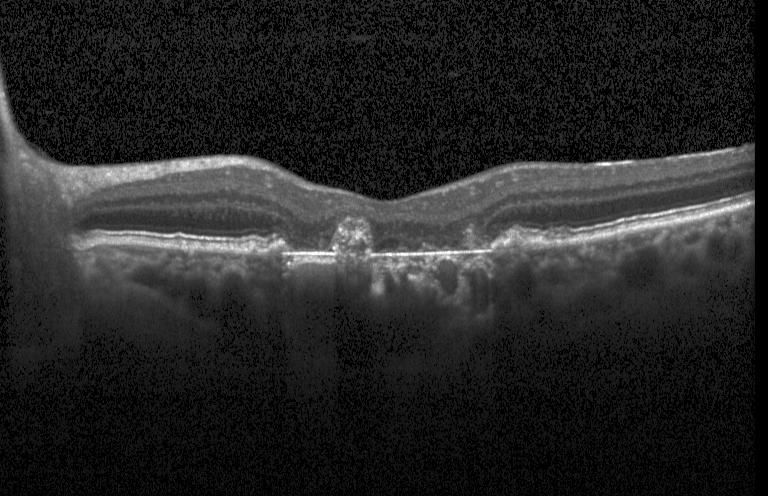 Dx: CNV.